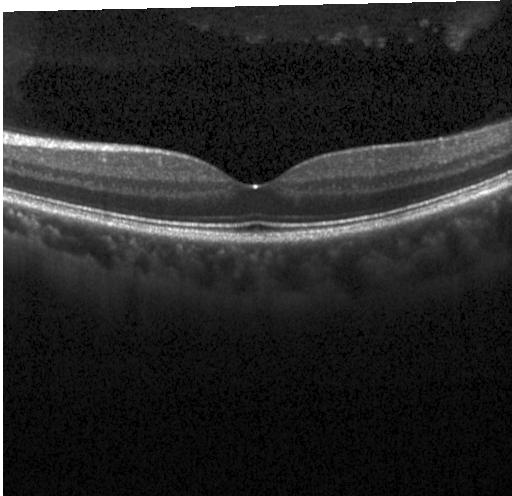

OCT scan showing neither choroidal neovascularization, diabetic macular edema, nor drusen.